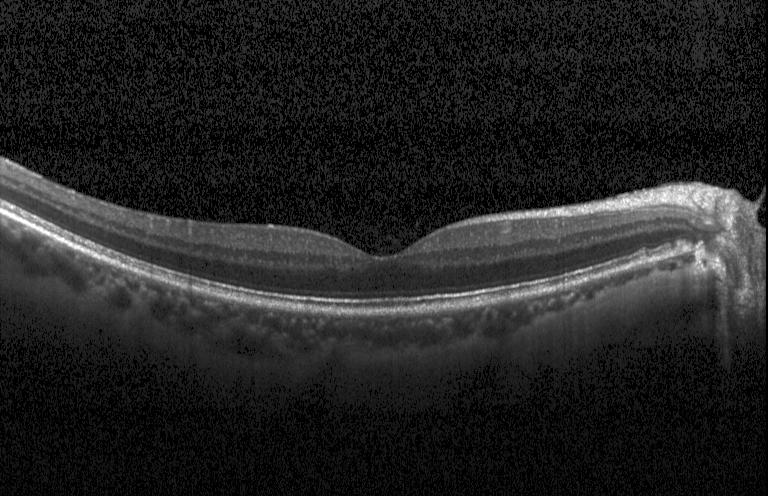 Retinal OCT cross-section
Macular OCT: no evidence of CNV, DME, or drusen.